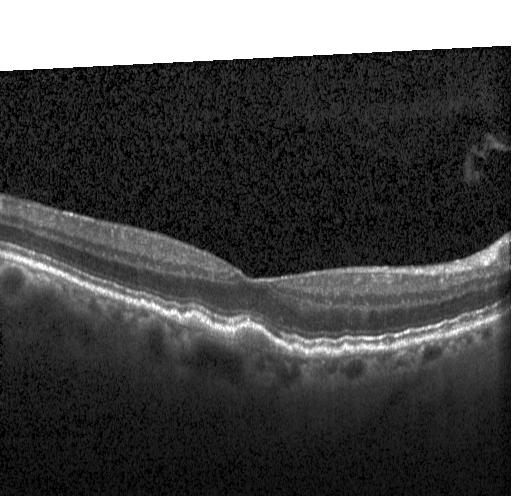
OCT B-scan showing CNV.